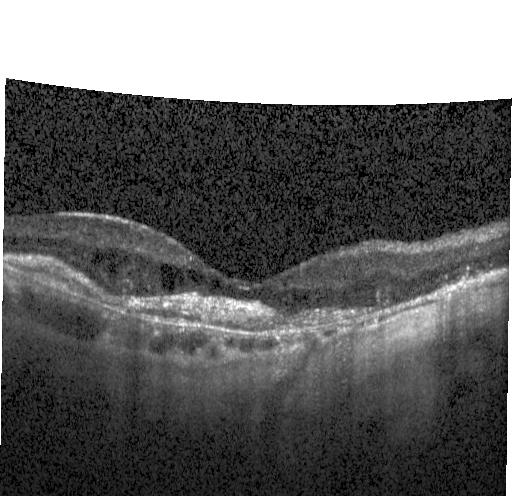 Retinal OCT cross-section showing choroidal neovascularization (CNV).